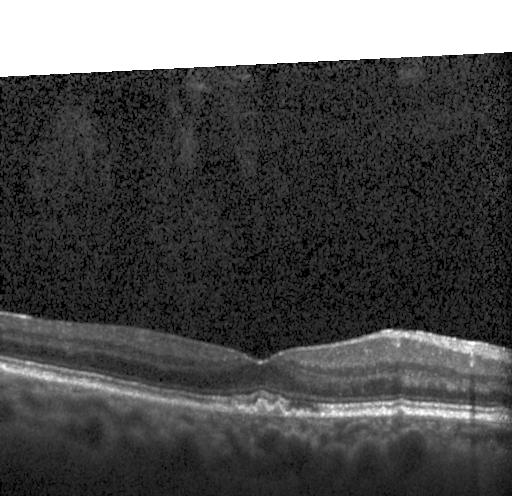 Macular OCT demonstrating multiple drusen.